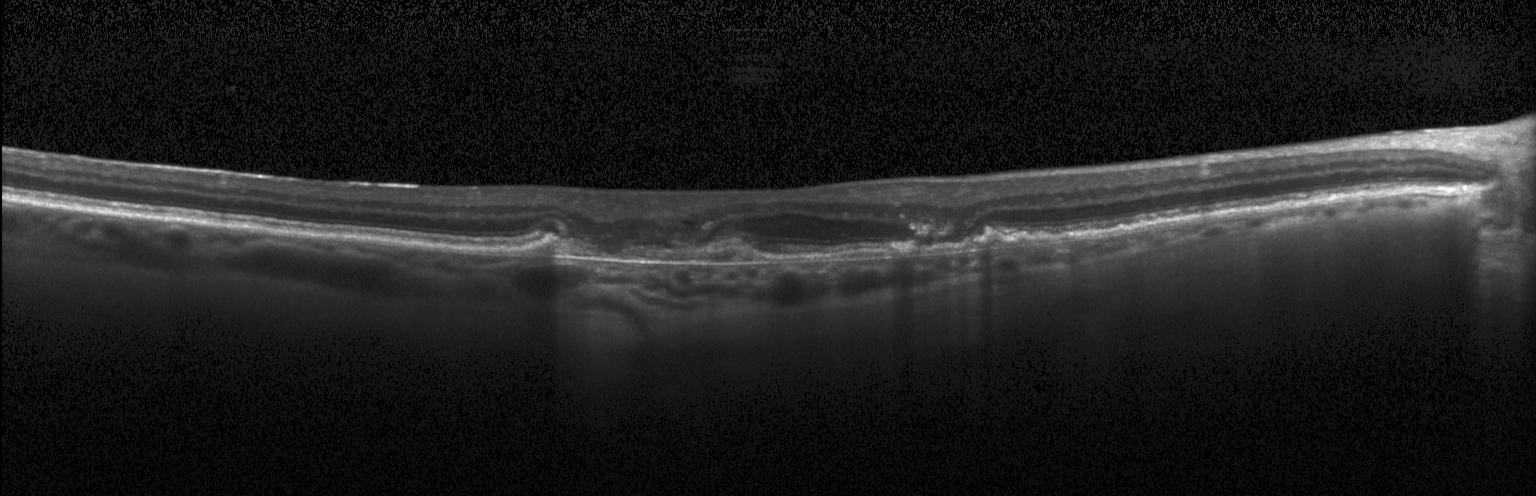 Optical coherence tomography B-scan
Macular OCT: a choroidal neovascular membrane.